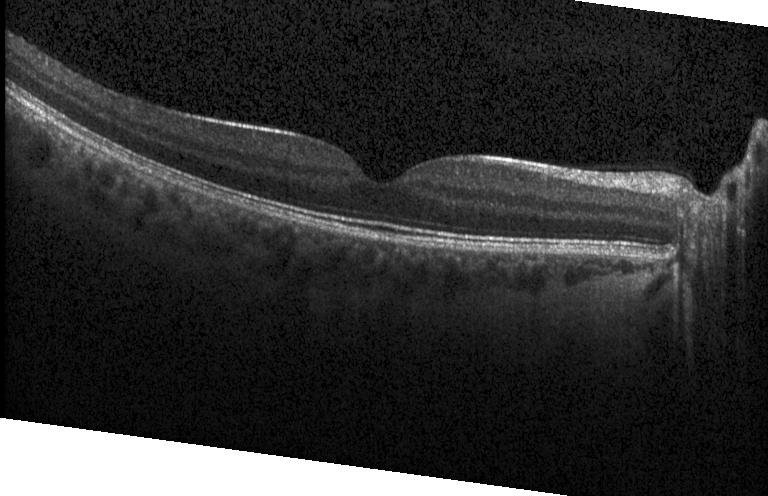
Impression: no CNV, DME, or drusen.